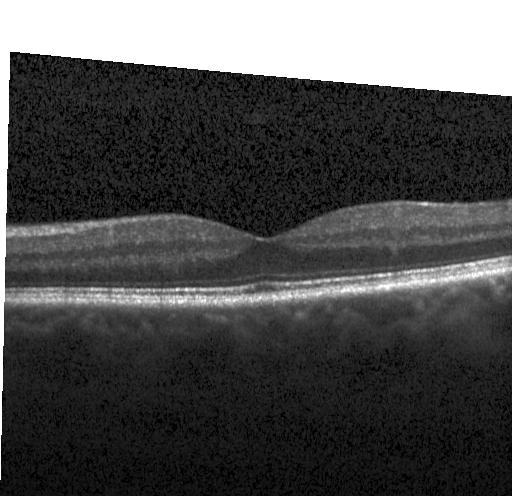 Optical coherence tomography B-scan — No evidence of choroidal neovascularization, diabetic macular edema, or drusen.